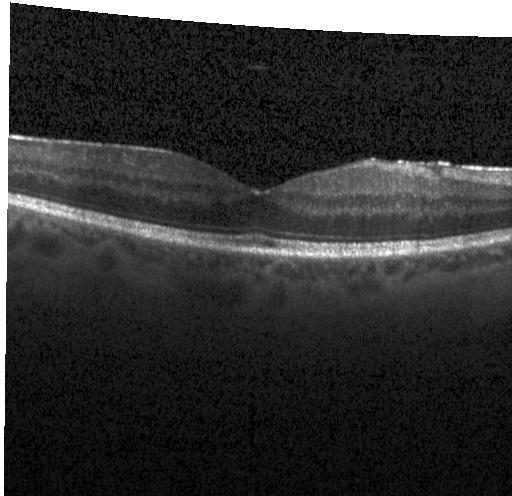
Retinal OCT B-scan. No choroidal neovascularization, diabetic macular edema, or drusen.